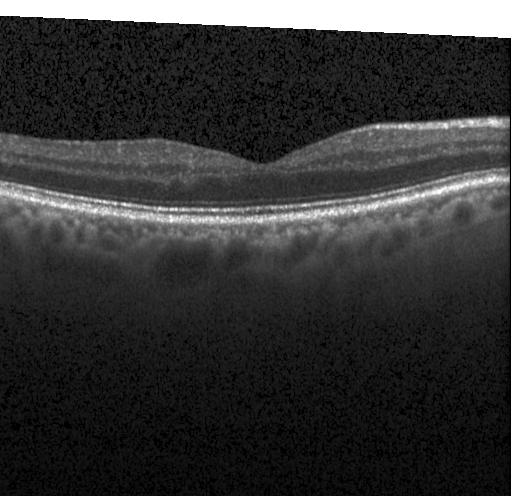 Heidelberg Spectralis OCT system, retinal OCT cross-section, spectral-domain OCT
Dx: no choroidal neovascularization, no diabetic macular edema, and no drusen.